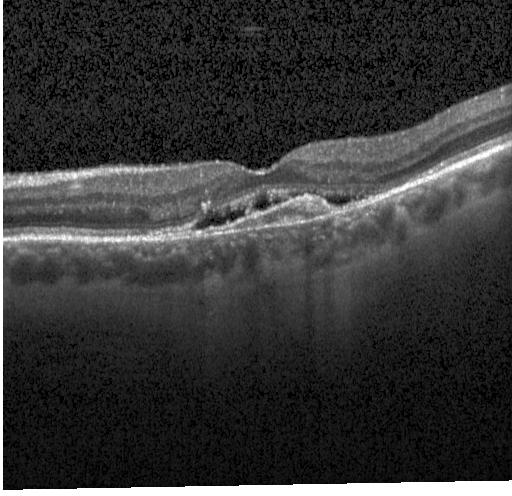

OCT line scan · centered on the fovea
OCT finding: choroidal neovascularization (CNV).